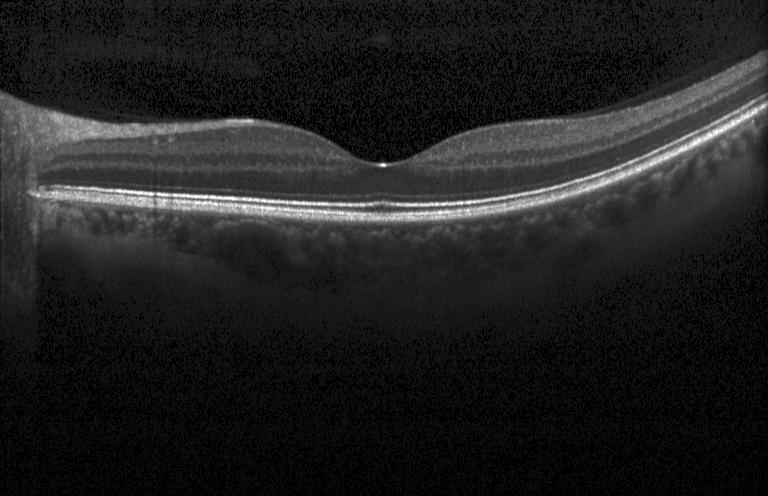 Acquired on a Heidelberg Spectralis, OCT B-scan.
Impression: neither CNV, DME, nor drusen.